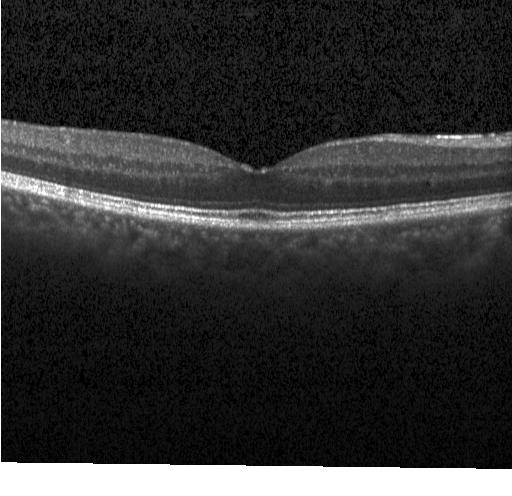 Heidelberg Spectralis, centered on the fovea, retinal OCT cross-section, spectral-domain optical coherence tomography.
Assessment: no CNV, no DME, and no drusen.